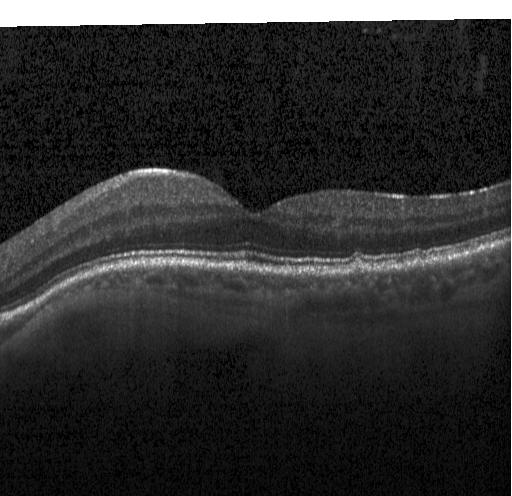
OCT line scan.
Finding: sub-RPE drusenoid deposits.